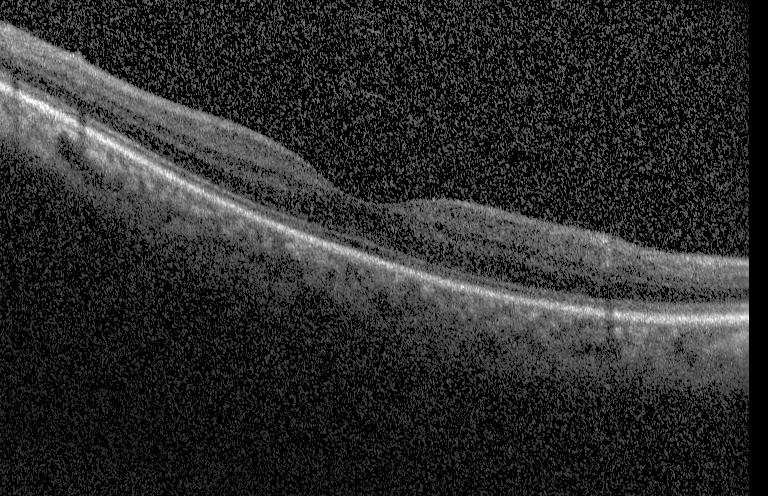

Spectral-domain optical coherence tomography. Instrument: Heidelberg Spectralis. Fovea-centered. OCT B-scan. No choroidal neovascularization, no diabetic macular edema, and no drusen.